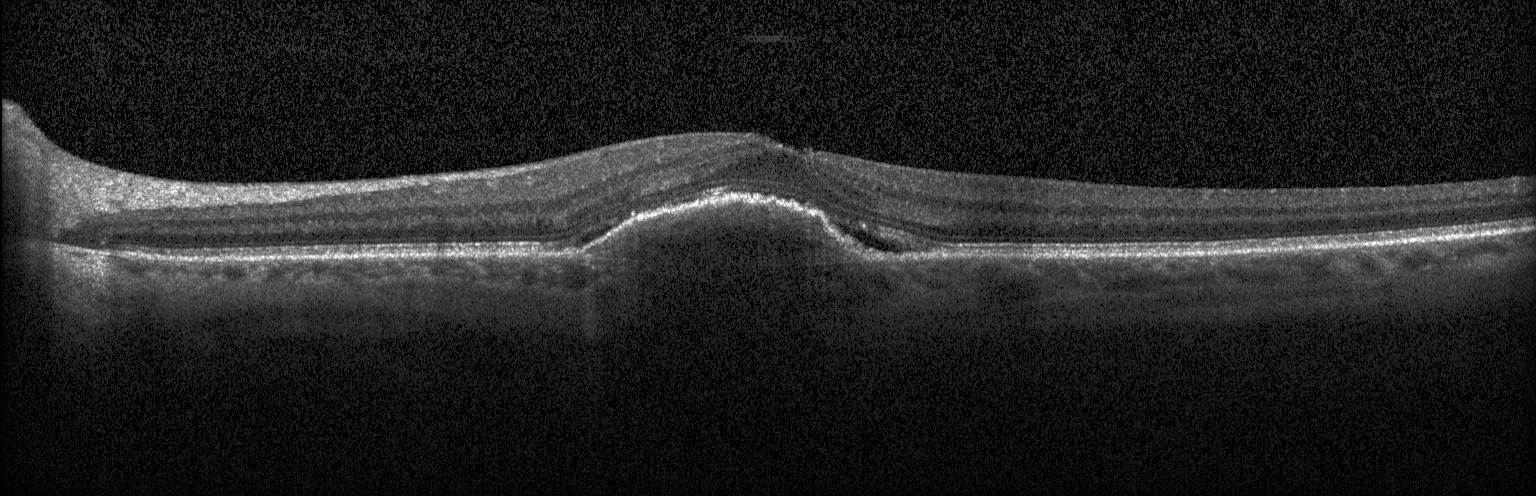

Finding: CNV.